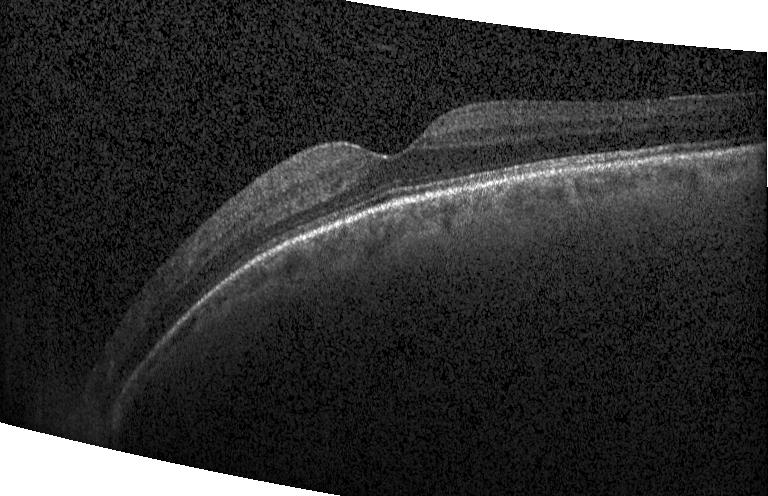

Fovea-centered · retinal OCT B-scan. The scan shows no evidence of CNV, DME, or drusen.